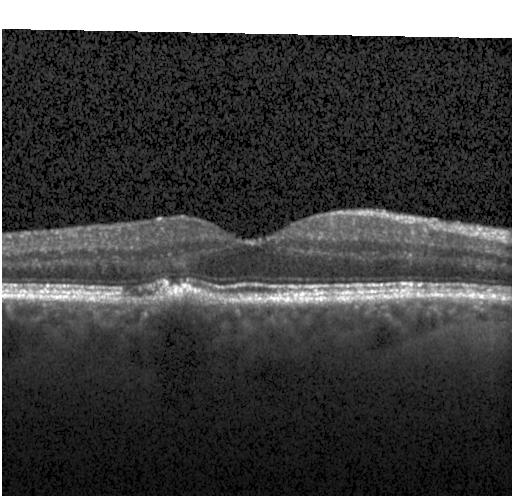 Optical coherence tomography B-scan
Assessment: drusen.